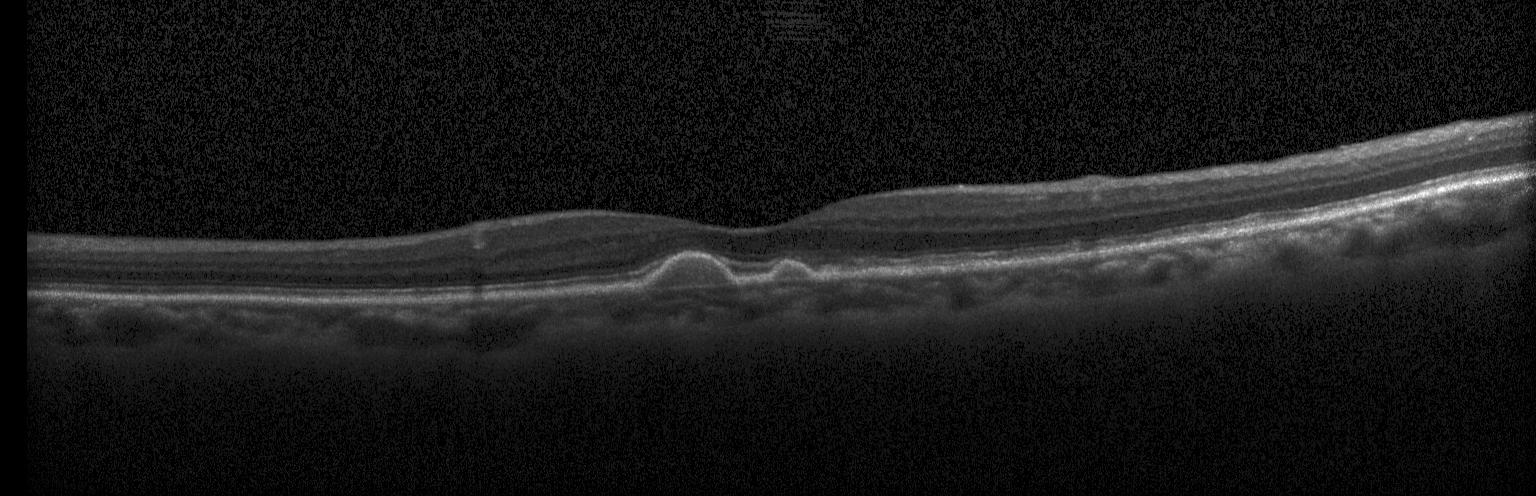

Macular OCT: drusen.